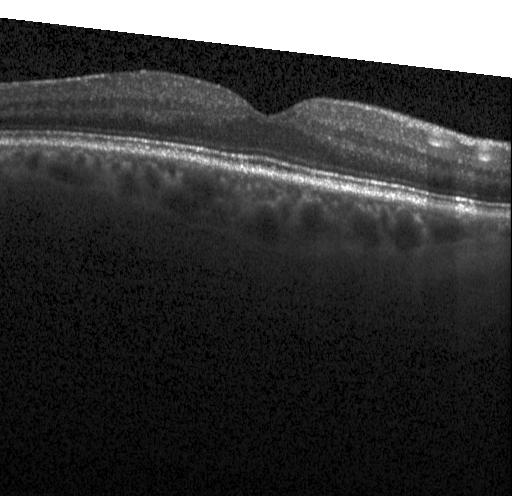 No choroidal neovascularization, diabetic macular edema, or drusen.